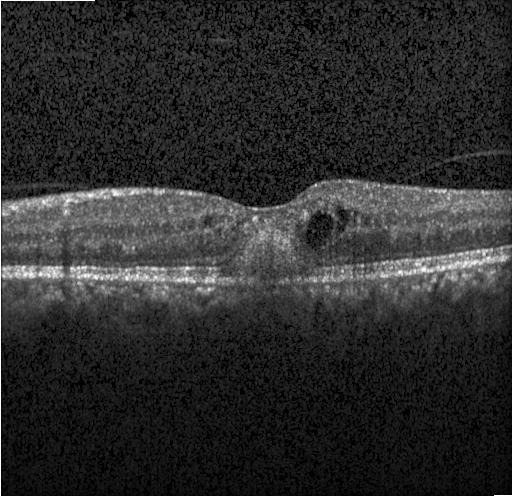 OCT B-scan. Centered on the fovea. SD-OCT. Heidelberg Spectralis OCT system. Macular OCT: choroidal neovascularization (CNV).